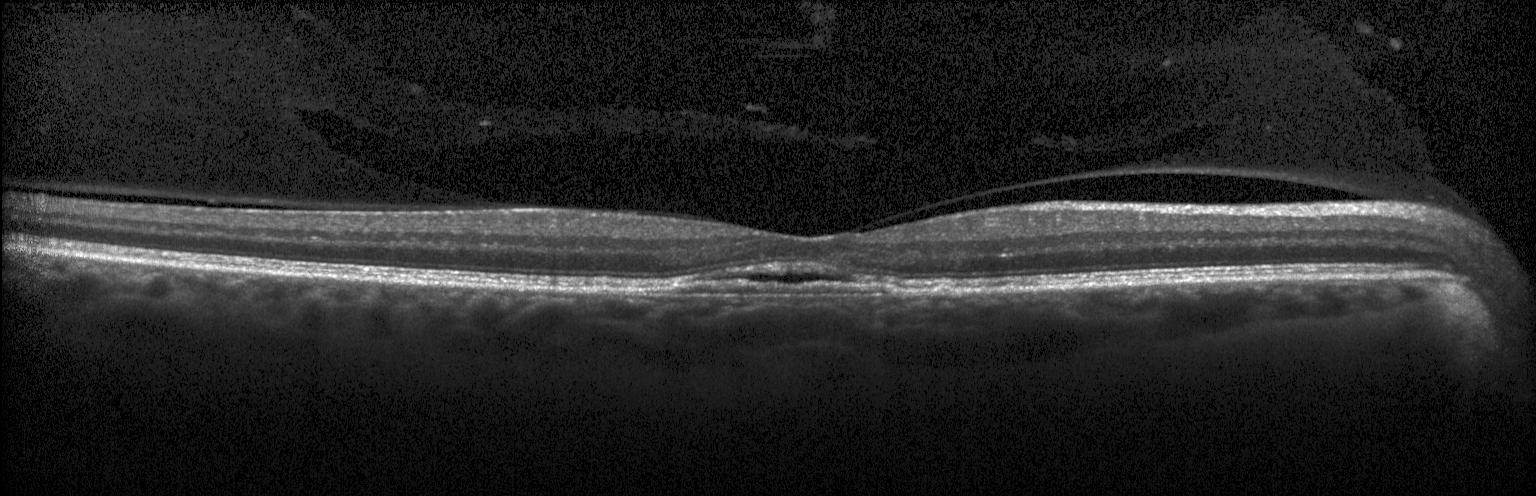 Retinal OCT B-scan; acquired on a Heidelberg Spectralis.
Assessment: CNV.